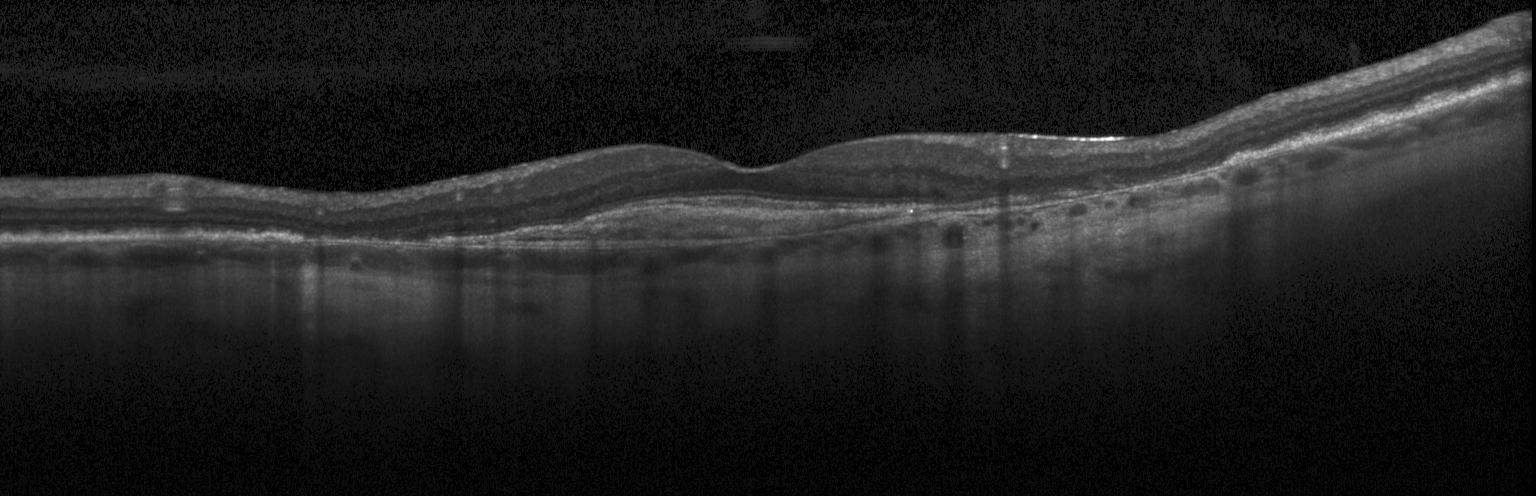
OCT B-scan showing choroidal neovascularization (CNV).